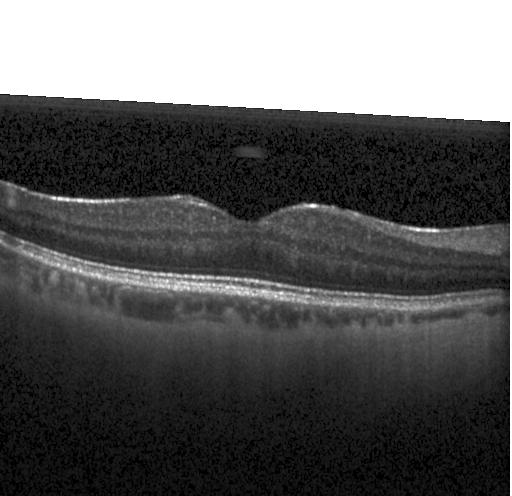 Spectral-domain OCT B-scan: no choroidal neovascularization, no diabetic macular edema, and no drusen.